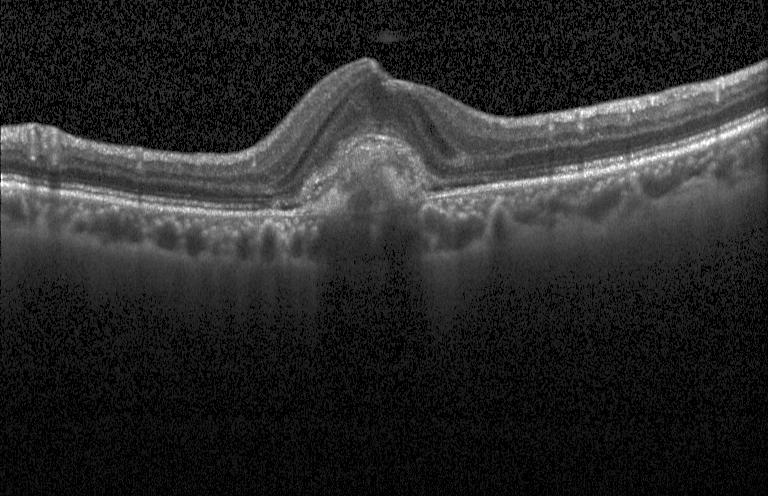 Optical coherence tomography scan, Heidelberg Spectralis OCT system, SD-OCT — Diagnosis: a choroidal neovascular membrane.